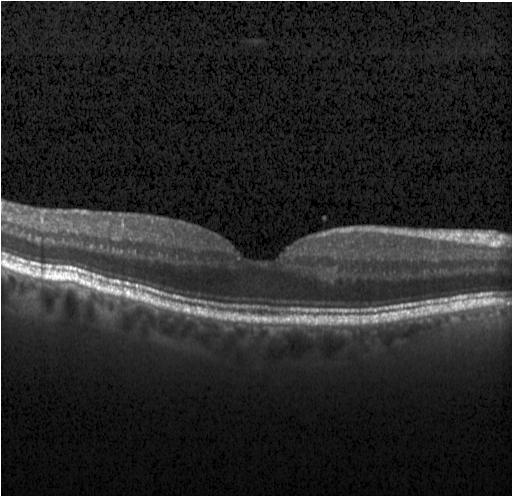

Retinal OCT B-scan; fovea-centered; spectral-domain optical coherence tomography; Heidelberg Spectralis.
This B-scan demonstrates no CNV, DME, or drusen.